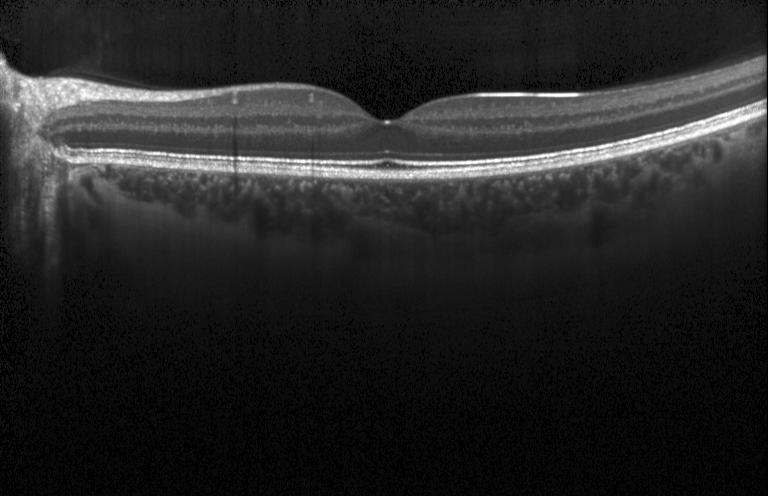

Fovea-centered. Retinal OCT cross-section — Impression: neither choroidal neovascularization, diabetic macular edema, nor drusen.